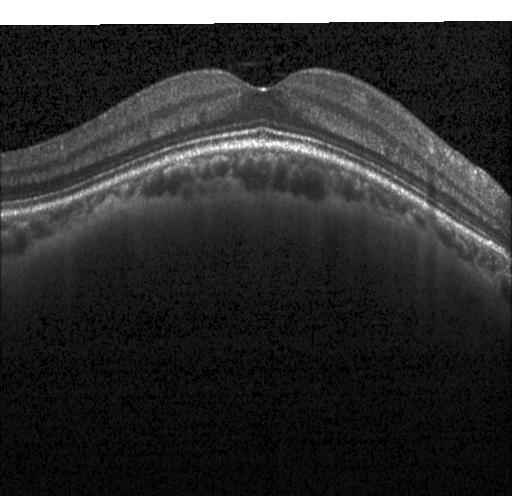 Macular scan. OCT line scan. SD-OCT. Dx: no choroidal neovascularization, no diabetic macular edema, and no drusen.